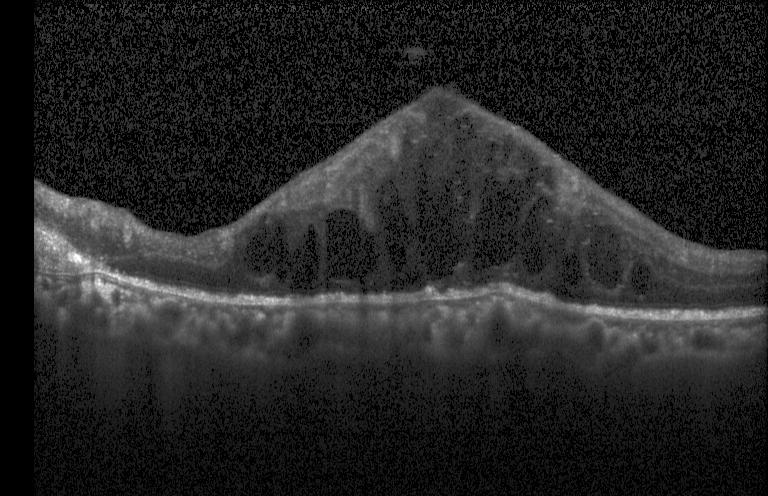

Retinal OCT B-scan — Dx: diabetic macular edema.